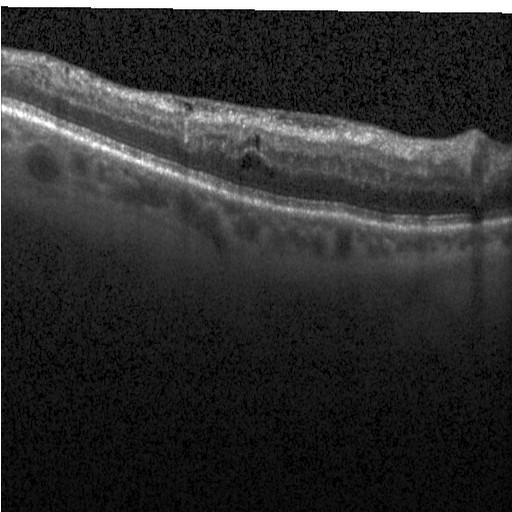

Diagnosis: diabetic macular edema (DME).